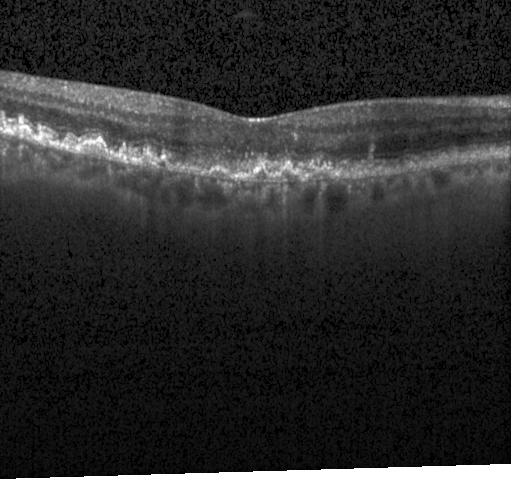 OCT finding: a choroidal neovascular membrane.